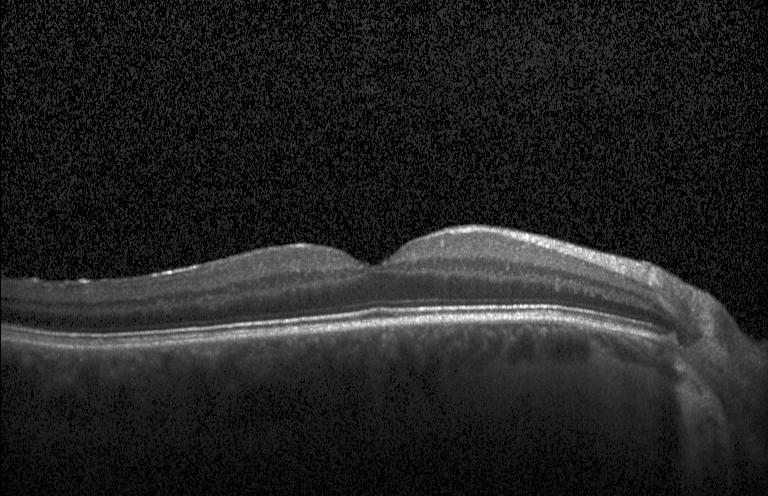

OCT B-scan — Impression: no CNV, no DME, and no drusen.